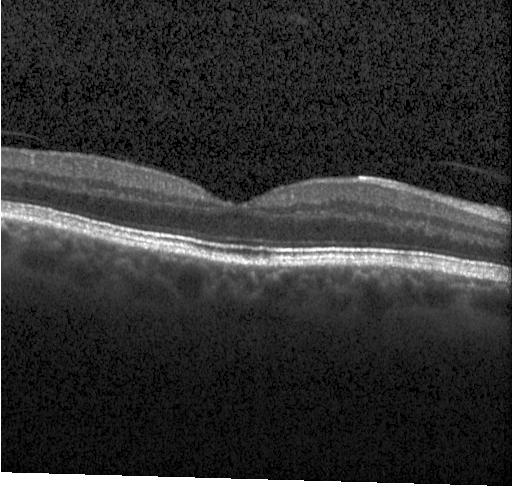
Finding: no choroidal neovascularization, diabetic macular edema, or drusen.